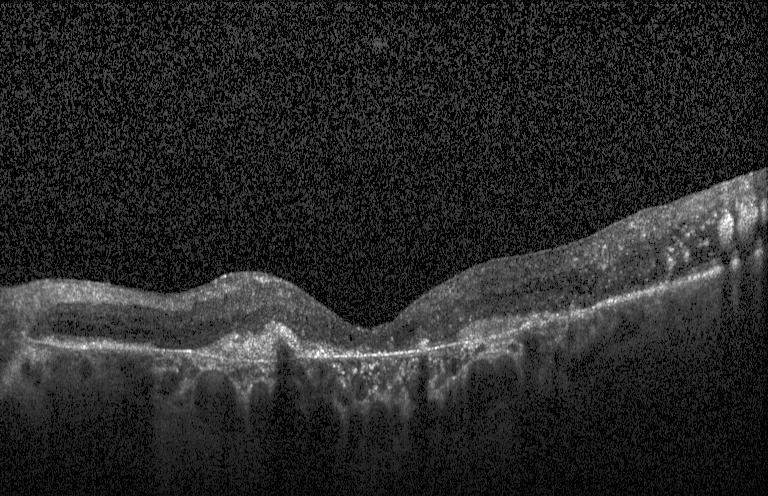
OCT B-scan, Heidelberg Spectralis, centered on the fovea — Diagnosis: CNV.